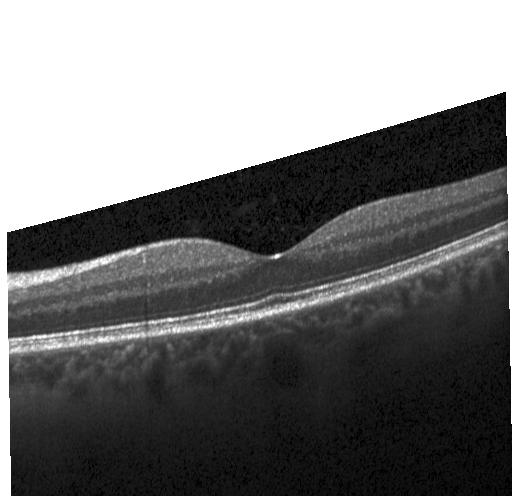 OCT finding: no evidence of choroidal neovascularization, diabetic macular edema, or drusen.